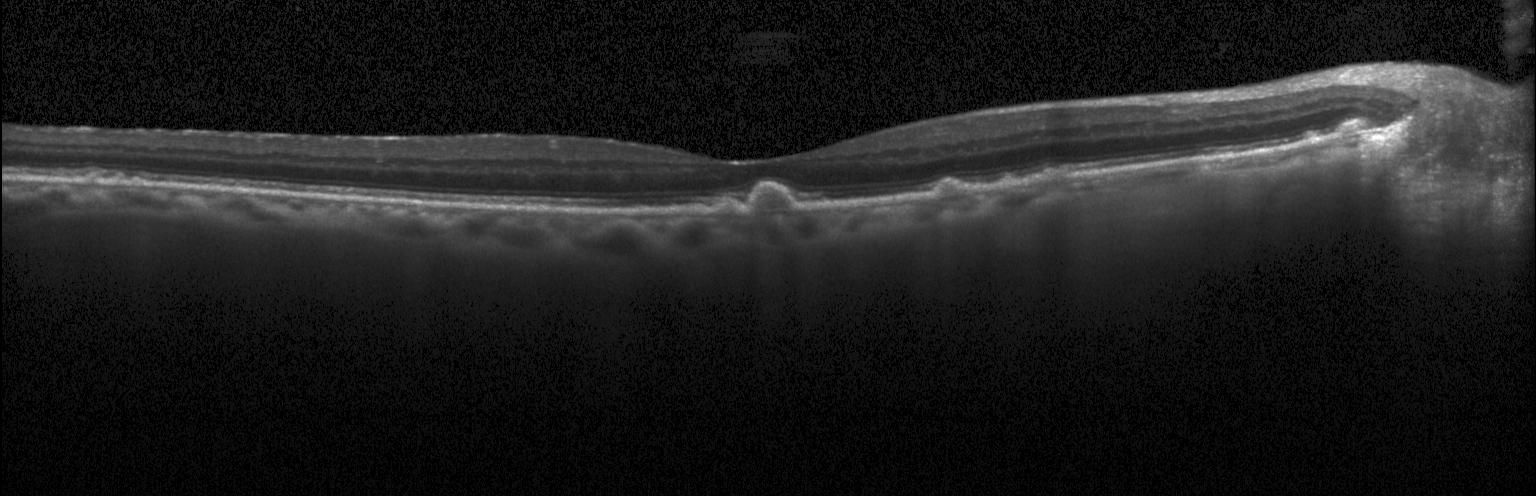
Spectral-domain OCT B-scan: multiple drusen.